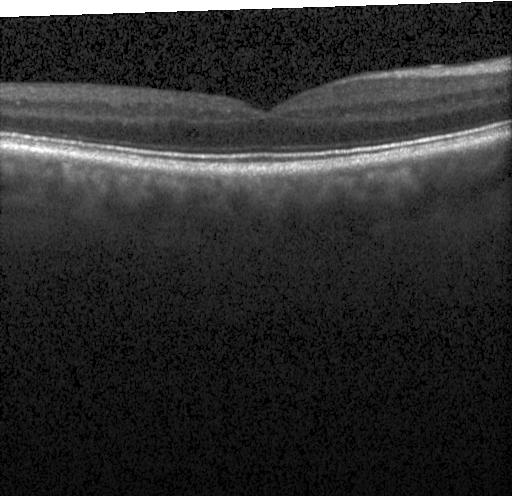

Macular scan. SD-OCT. OCT line scan. Heidelberg Spectralis OCT system. Impression: no choroidal neovascularization, no diabetic macular edema, and no drusen.